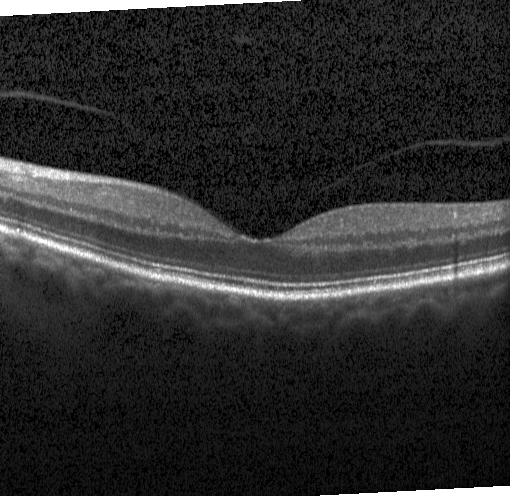

OCT B-scan. Instrument: Heidelberg Spectralis. SD-OCT. Fovea-centered.
Diagnosis: no choroidal neovascularization, no diabetic macular edema, and no drusen.